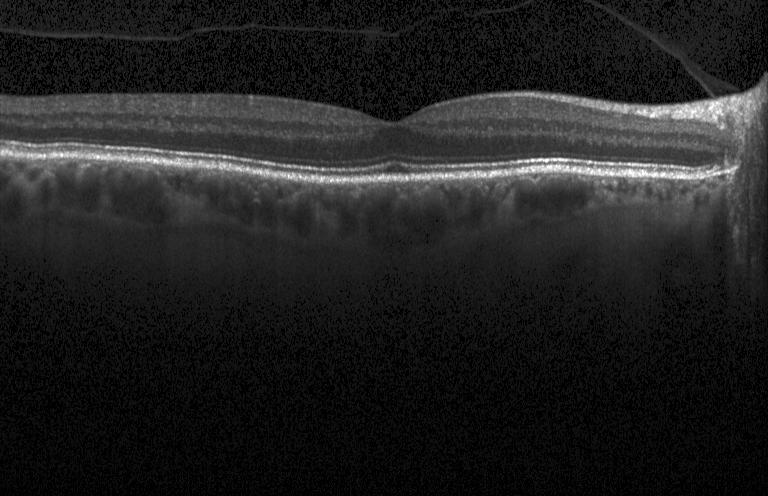 Retinal OCT cross-section showing no choroidal neovascularization, diabetic macular edema, or drusen.